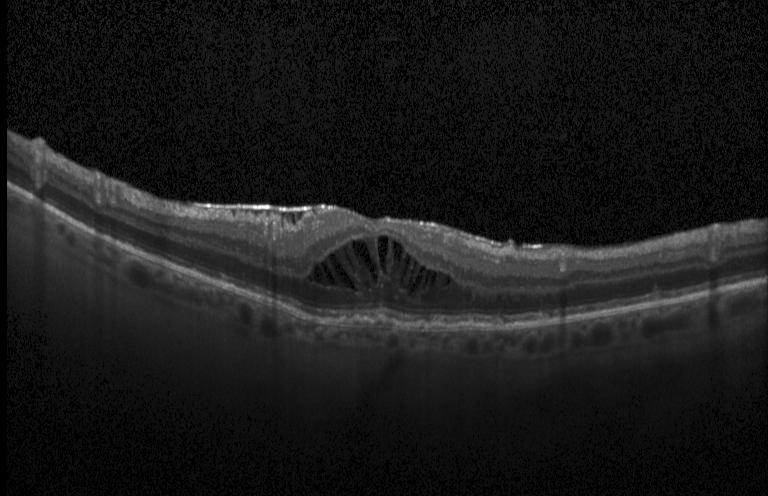
Impression: diabetic macular edema.